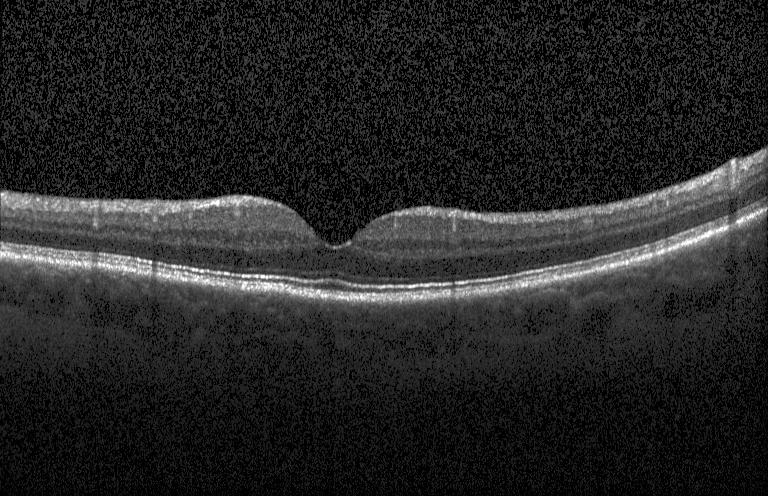 Through the macula; retinal OCT cross-section; instrument: Heidelberg Spectralis; SD-OCT.
Finding: neither CNV, DME, nor drusen.